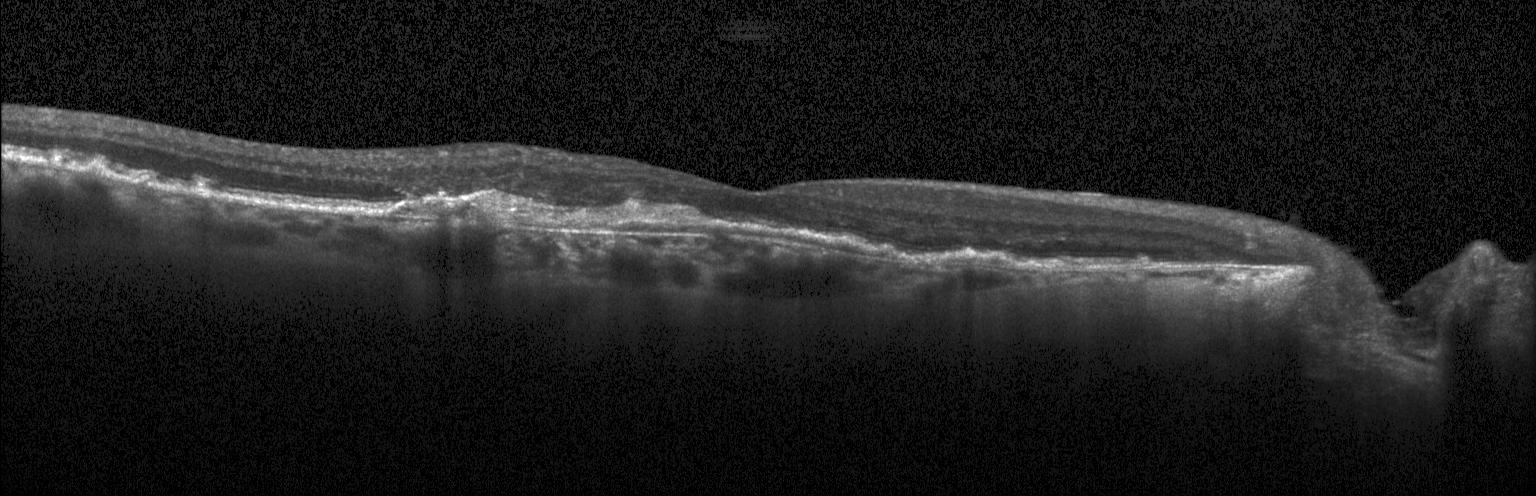 Centered on the fovea · Heidelberg Spectralis · spectral-domain OCT · OCT line scan.
Diagnosis: a choroidal neovascular membrane.